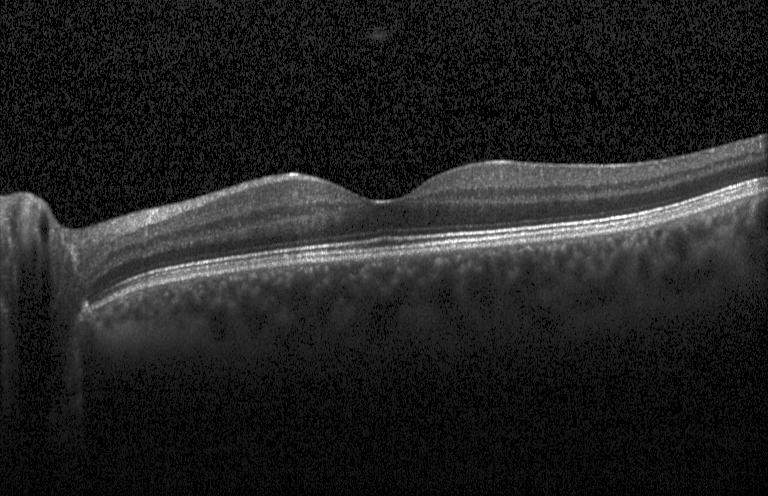 OCT scan showing no evidence of CNV, DME, or drusen.